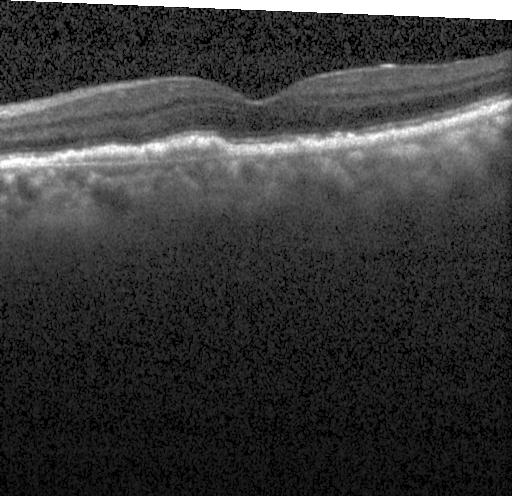

Fovea-centered · optical coherence tomography B-scan · spectral-domain optical coherence tomography · Heidelberg Spectralis OCT system
Finding: a choroidal neovascular membrane.